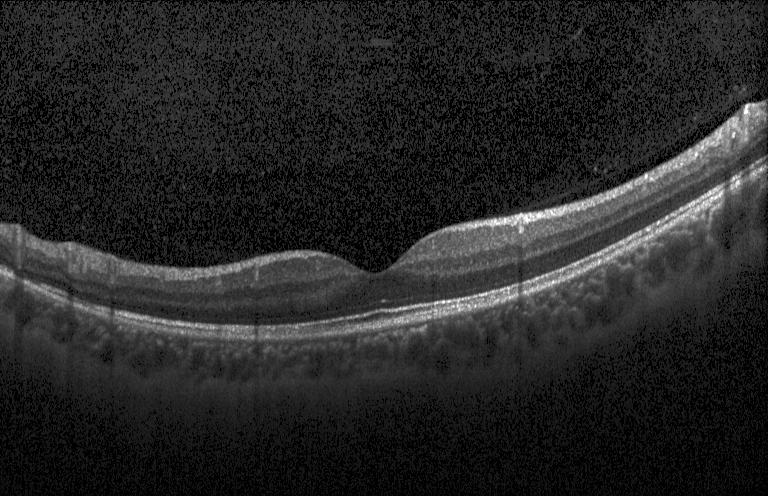

Retinal OCT cross-section, horizontal scan through the fovea
This B-scan demonstrates no evidence of choroidal neovascularization, diabetic macular edema, or drusen.